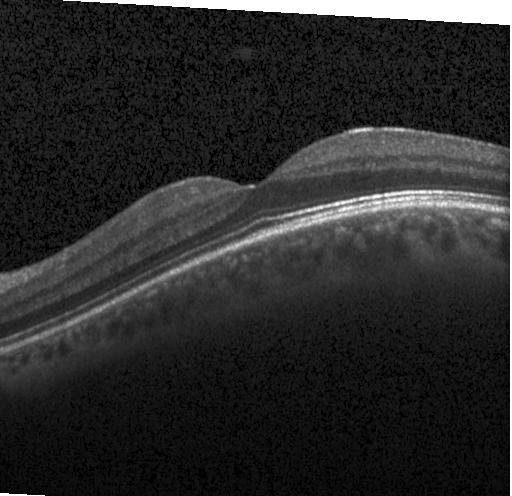
Retinal OCT cross-section showing no evidence of choroidal neovascularization, diabetic macular edema, or drusen.